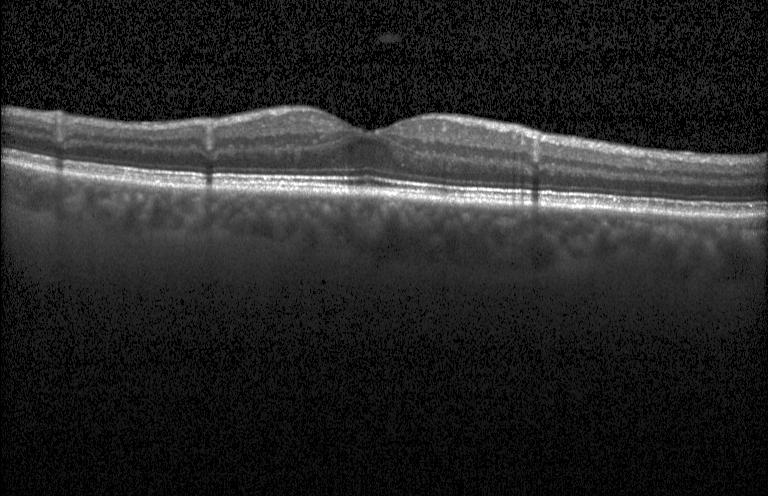

SD-OCT · Heidelberg Spectralis OCT system · horizontal scan through the fovea · optical coherence tomography B-scan. Dx: no choroidal neovascularization, diabetic macular edema, or drusen.